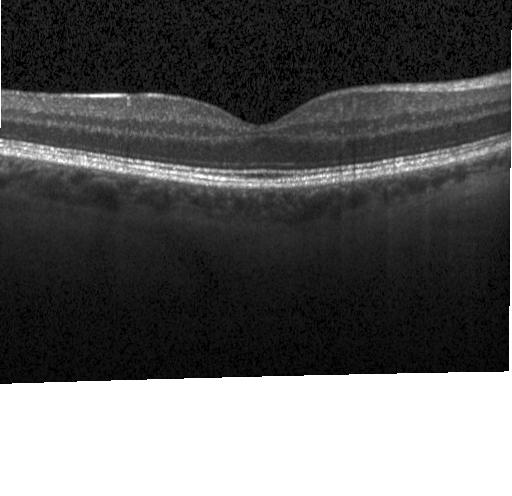
Diagnosis: no evidence of choroidal neovascularization, diabetic macular edema, or drusen.